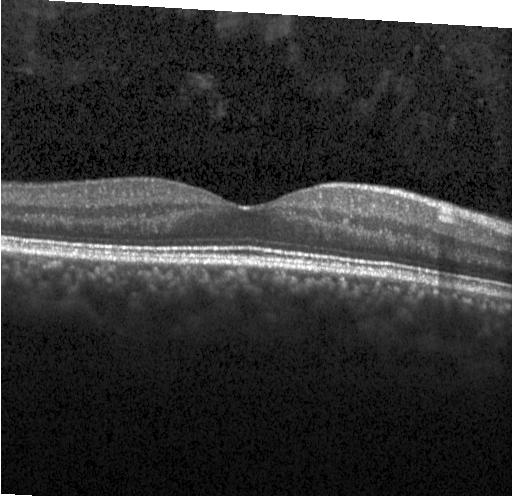

Optical coherence tomography B-scan. The scan shows neither choroidal neovascularization, diabetic macular edema, nor drusen.